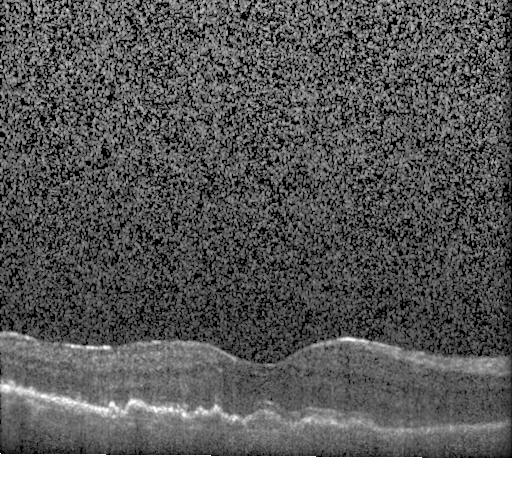 OCT scan showing choroidal neovascularization (CNV).